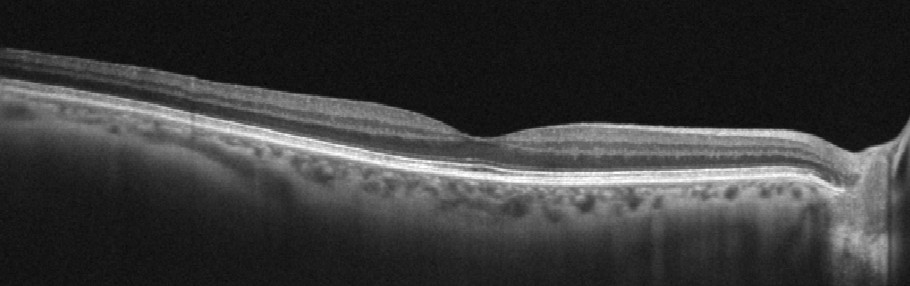

Through the macula; OCT line scan — Diagnosis: no evidence of AMD, DME, ERM, RAO, RVO, or VID.